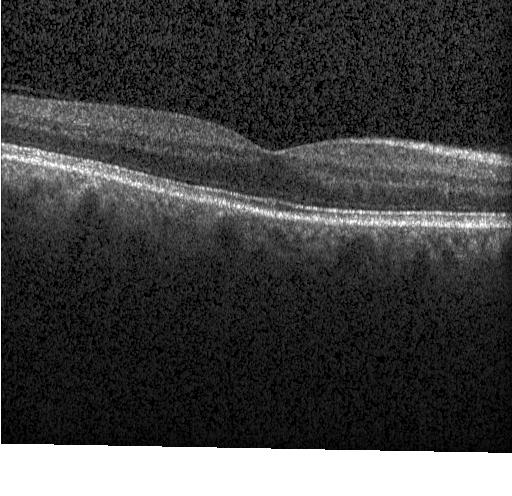
Optical coherence tomography B-scan · acquired on a Heidelberg Spectralis · horizontal scan through the fovea.
Finding: no choroidal neovascularization, diabetic macular edema, or drusen.